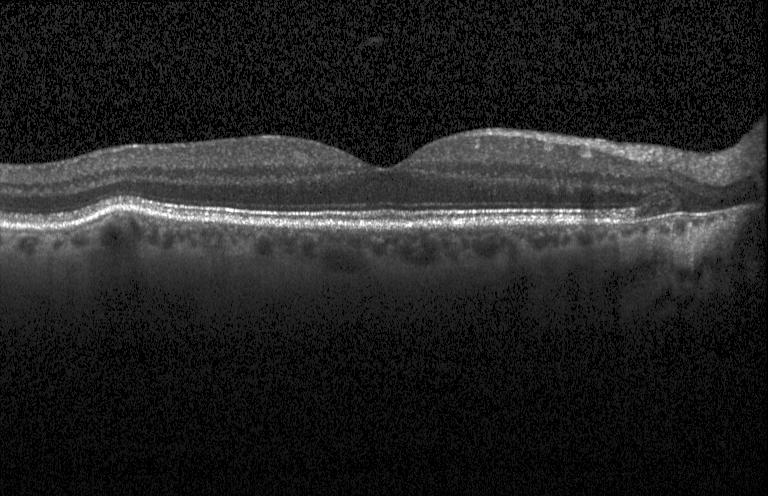

Heidelberg Spectralis, horizontal scan through the fovea, spectral-domain optical coherence tomography, OCT B-scan
Finding: no choroidal neovascularization, no diabetic macular edema, and no drusen.